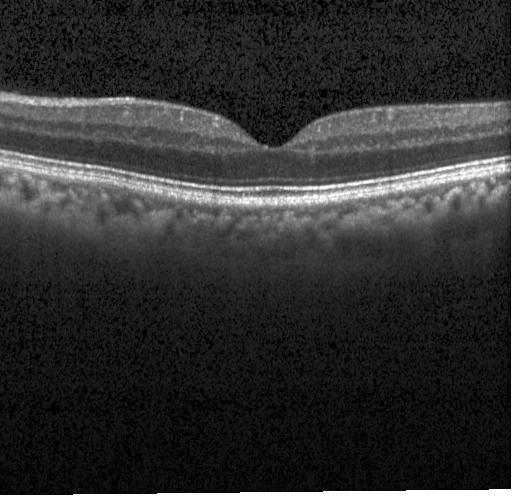
Optical coherence tomography scan. Diagnosis: no choroidal neovascularization, no diabetic macular edema, and no drusen.